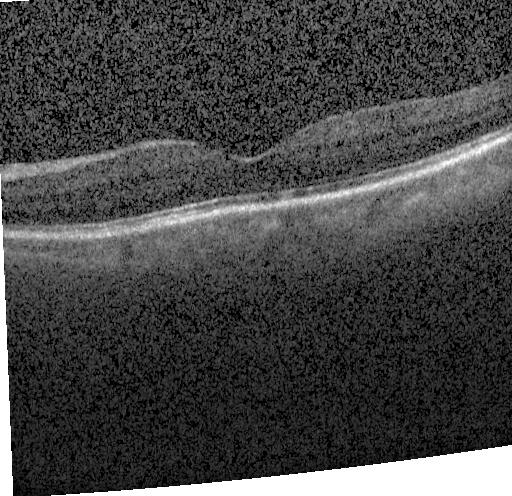 Macular OCT: no choroidal neovascularization, no diabetic macular edema, and no drusen.